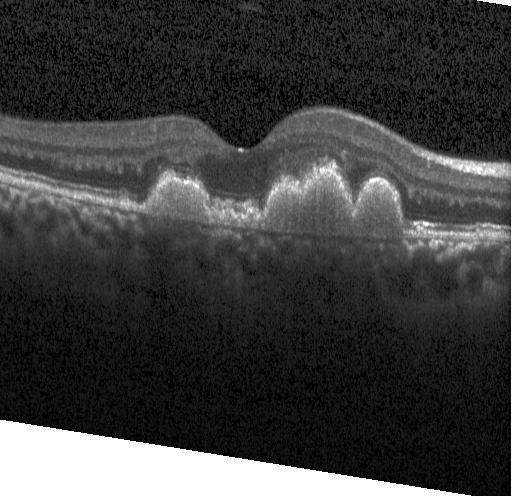 Heidelberg Spectralis OCT system, retinal OCT cross-section — This B-scan demonstrates sub-RPE drusenoid deposits.